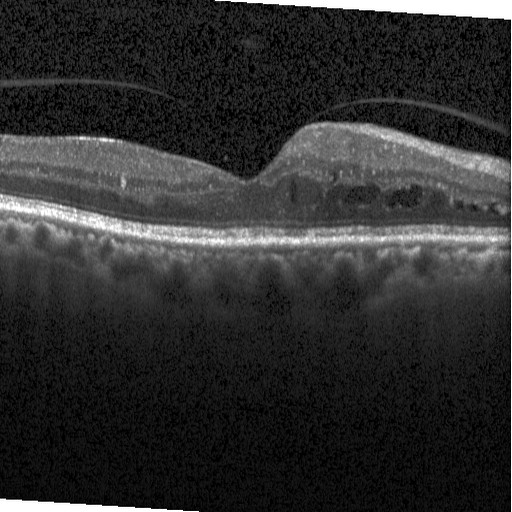

Finding: DME.